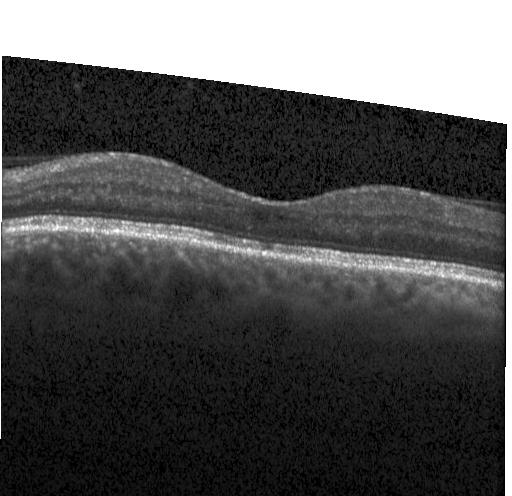 Heidelberg Spectralis; SD-OCT; retinal OCT B-scan; centered on the fovea — No evidence of choroidal neovascularization, diabetic macular edema, or drusen.